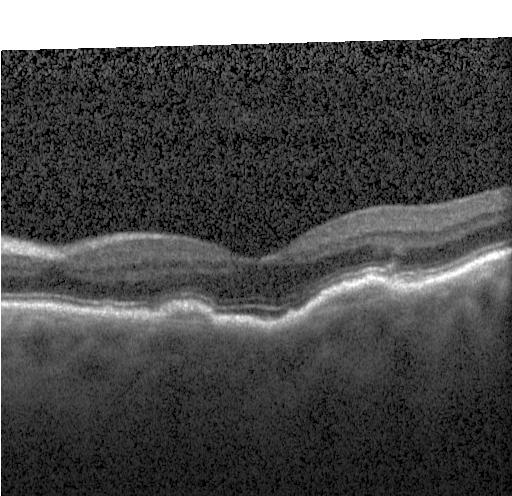

OCT line scan — Diagnosis: choroidal neovascularization (CNV).